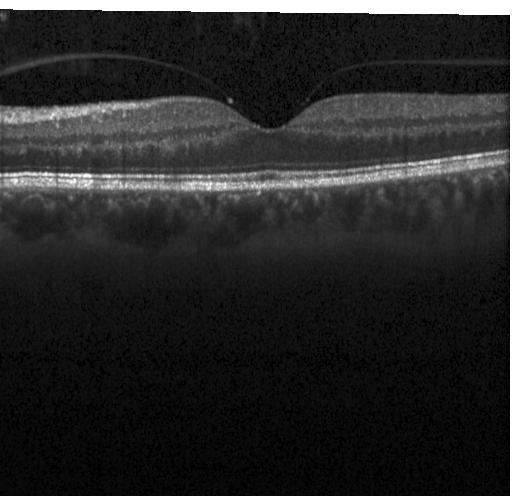
Optical coherence tomography B-scan. Finding: neither choroidal neovascularization, diabetic macular edema, nor drusen.